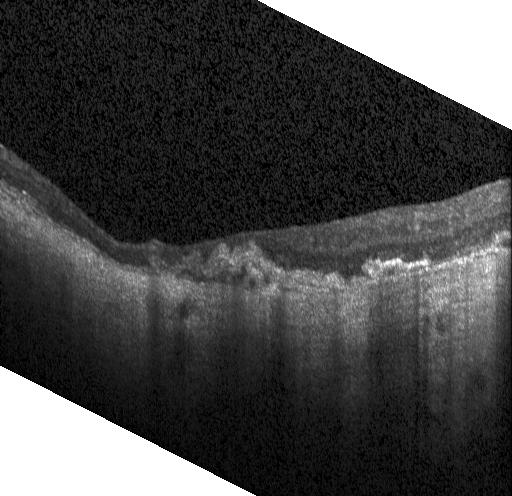 OCT finding: CNV.